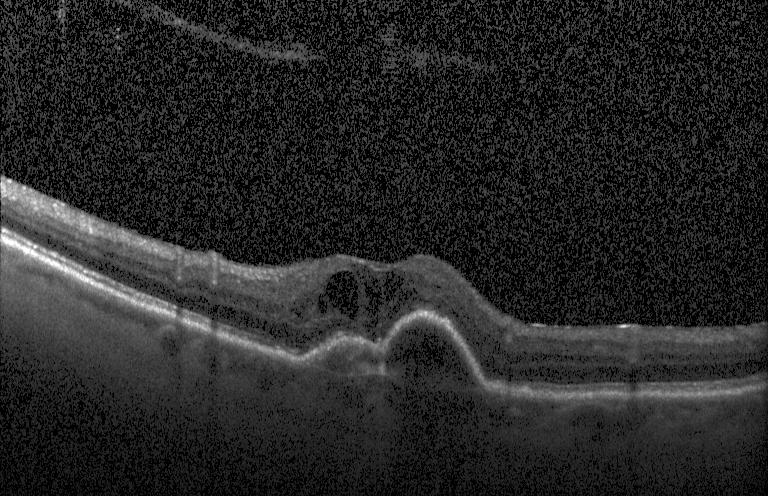
Optical coherence tomography B-scan — Dx: choroidal neovascularization.